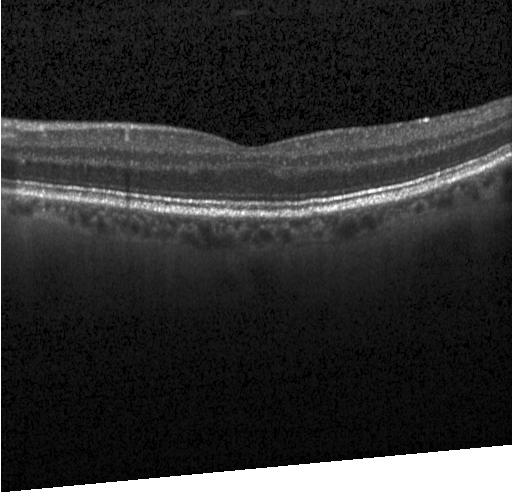
Diagnosis: no evidence of CNV, DME, or drusen.